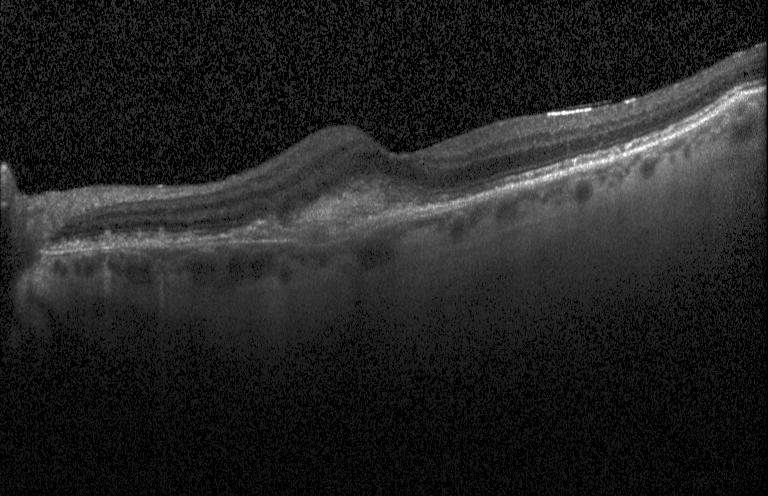
Retinal OCT cross-section.
Impression: a choroidal neovascular membrane.